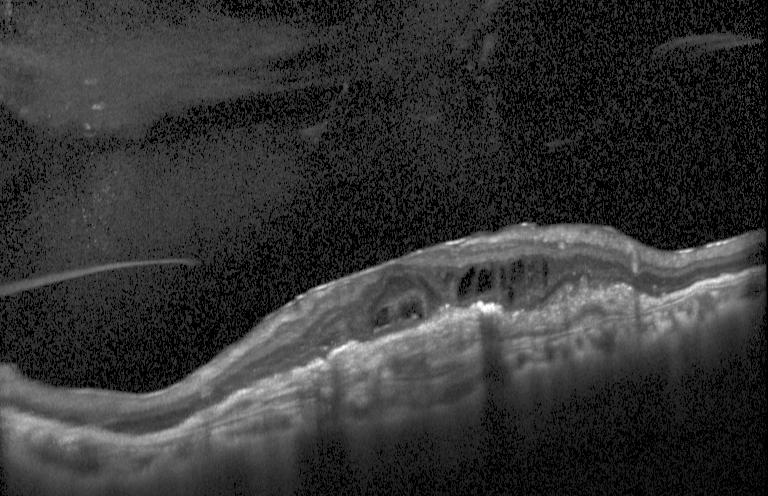

Diagnosis: a choroidal neovascular membrane.